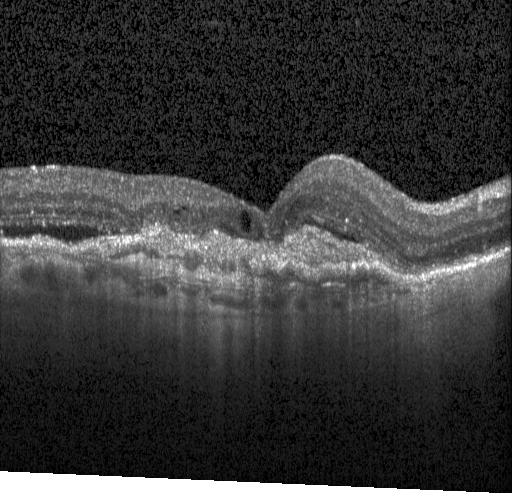

OCT B-scan showing a choroidal neovascular membrane.